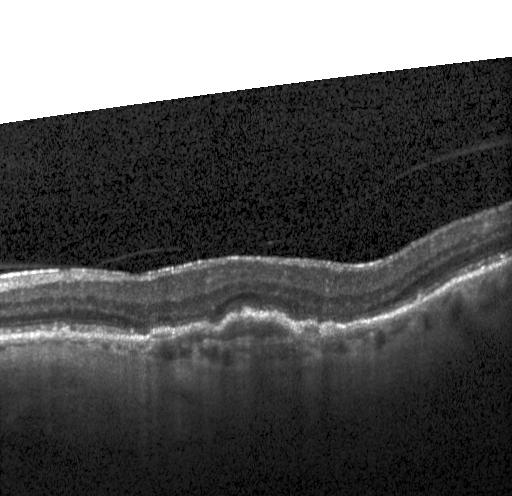 Impression: choroidal neovascularization.